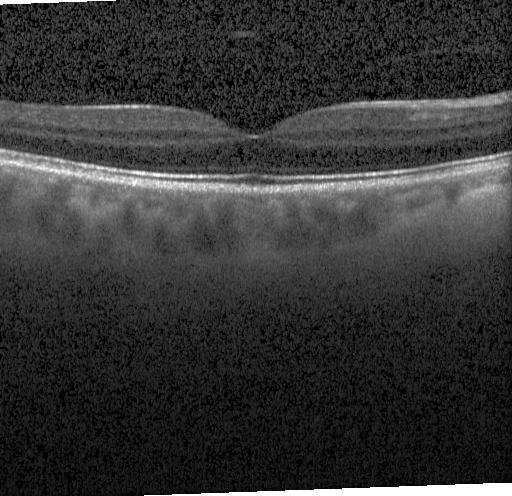

OCT B-scan; spectral-domain optical coherence tomography; through the macula; instrument: Heidelberg Spectralis.
Macular OCT: no evidence of CNV, DME, or drusen.